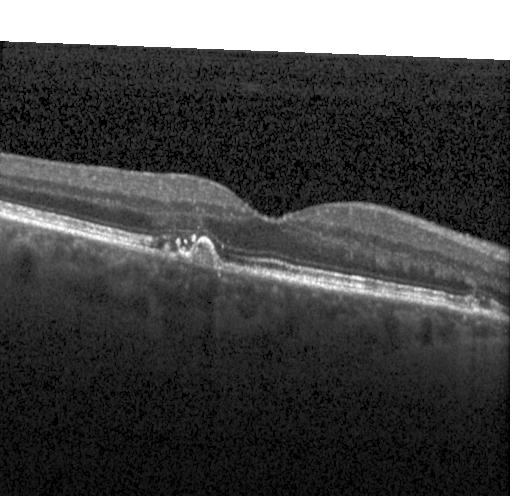 Optical coherence tomography scan, through the macula, Heidelberg Spectralis OCT system — Diagnosis: choroidal neovascularization (CNV).